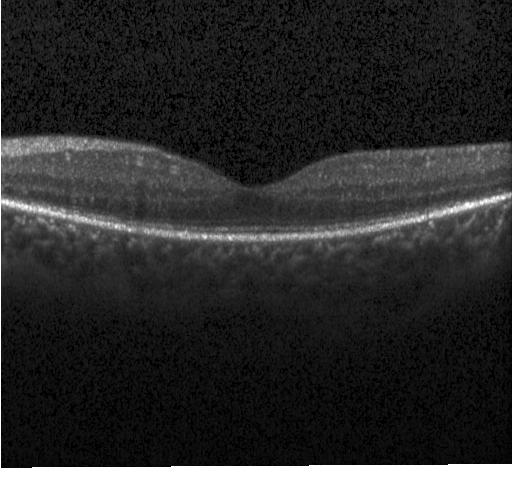
Optical coherence tomography scan — Finding: no evidence of CNV, DME, or drusen.